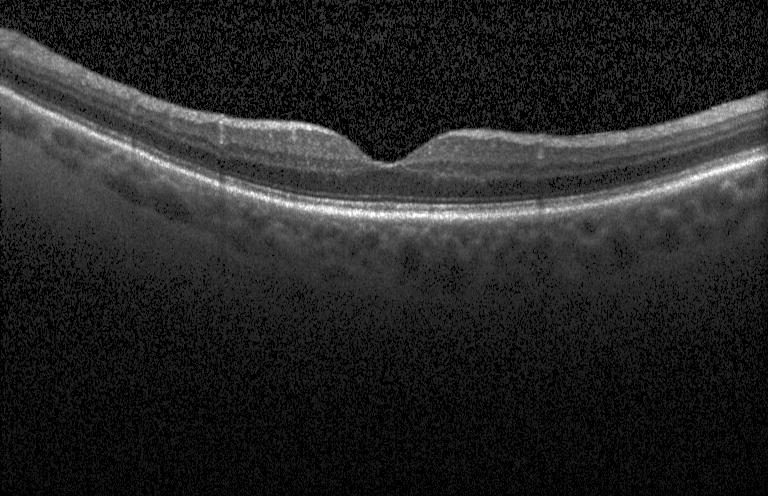
Retinal OCT B-scan · instrument: Heidelberg Spectralis.
Impression: no CNV, DME, or drusen.